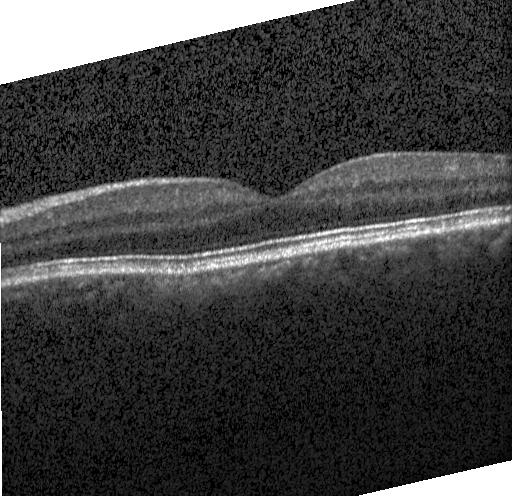
Heidelberg Spectralis OCT system · optical coherence tomography scan
OCT finding: no choroidal neovascularization, no diabetic macular edema, and no drusen.